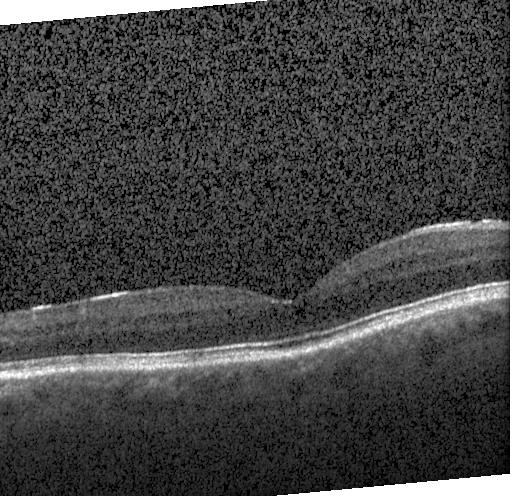

Finding: no choroidal neovascularization, diabetic macular edema, or drusen.